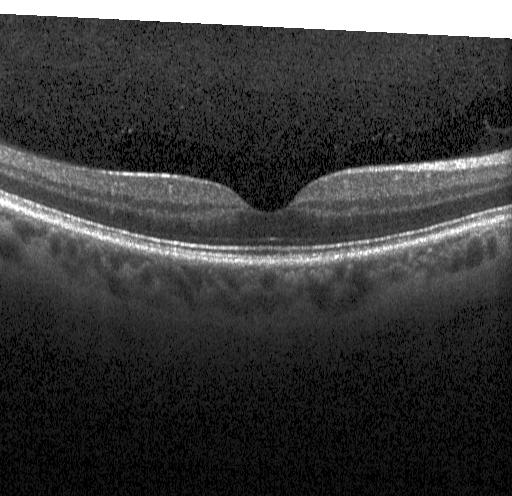

Diagnosis: no choroidal neovascularization, no diabetic macular edema, and no drusen.